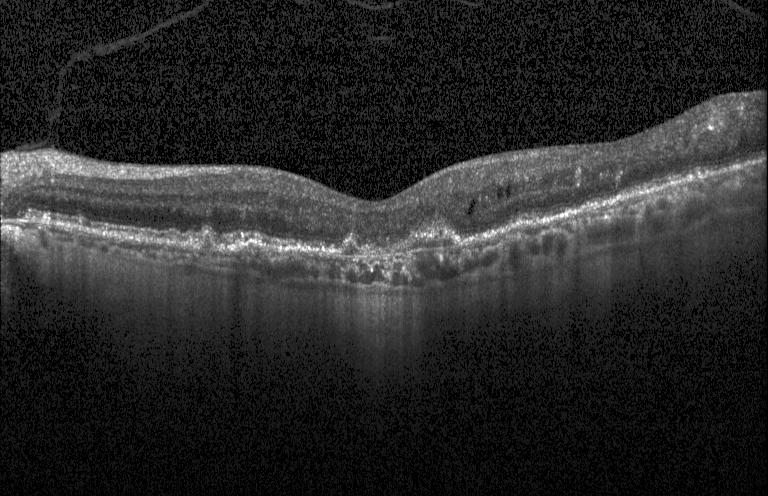
Optical coherence tomography scan.
Impression: CNV.